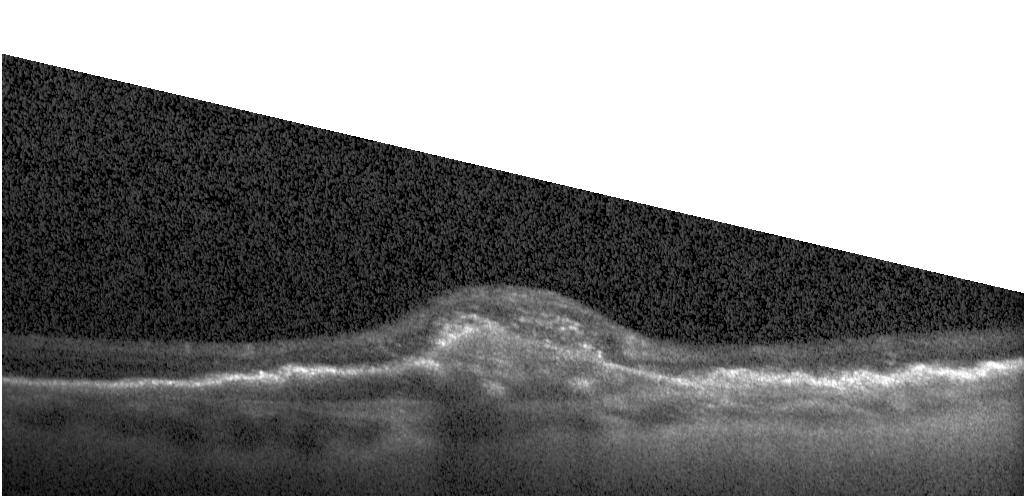

Optical coherence tomography B-scan
This B-scan demonstrates choroidal neovascularization (CNV).